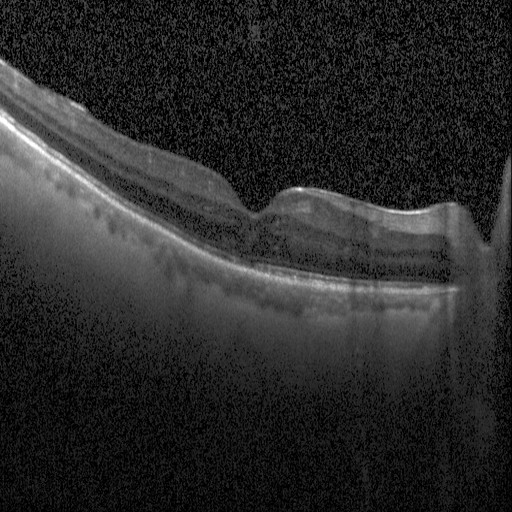

Optical coherence tomography B-scan. Assessment: DME.